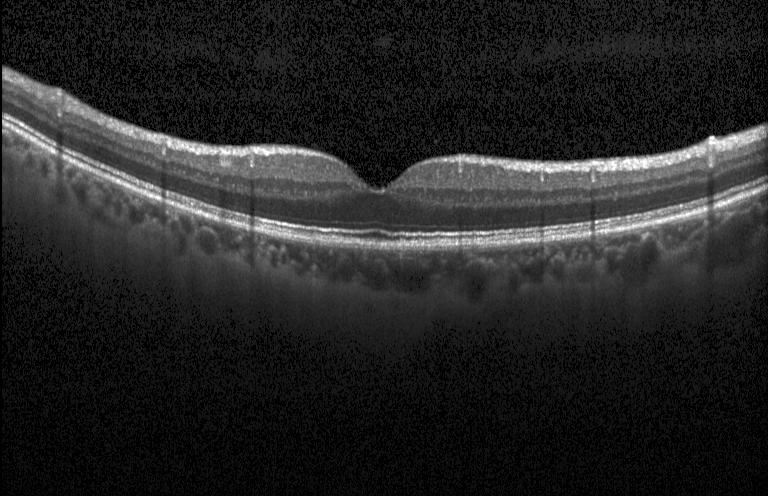 Macular scan · Heidelberg Spectralis · optical coherence tomography scan · SD-OCT
The scan shows neither CNV, DME, nor drusen.